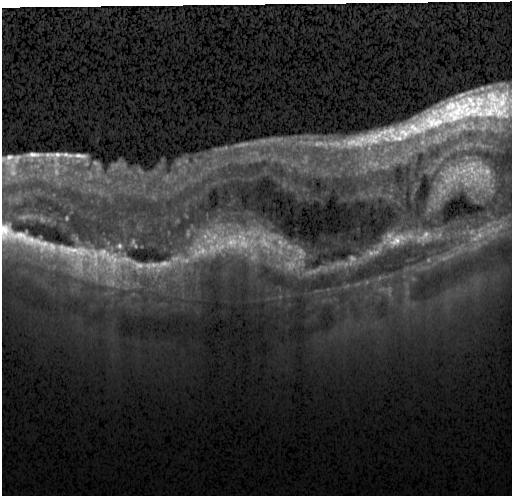

Macular scan. Optical coherence tomography B-scan. Heidelberg Spectralis. Spectral-domain OCT.
Assessment: a choroidal neovascular membrane.